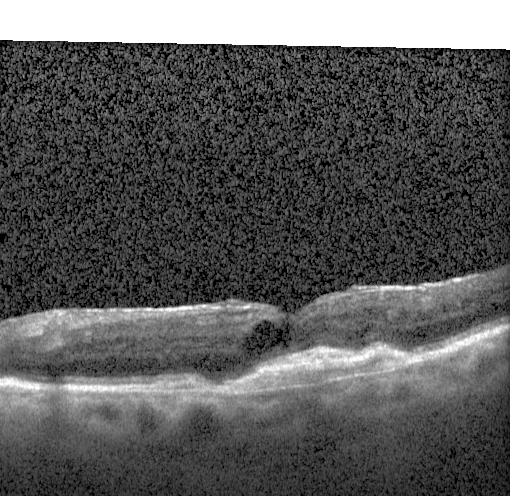 Retinal OCT B-scan
Assessment: a choroidal neovascular membrane.